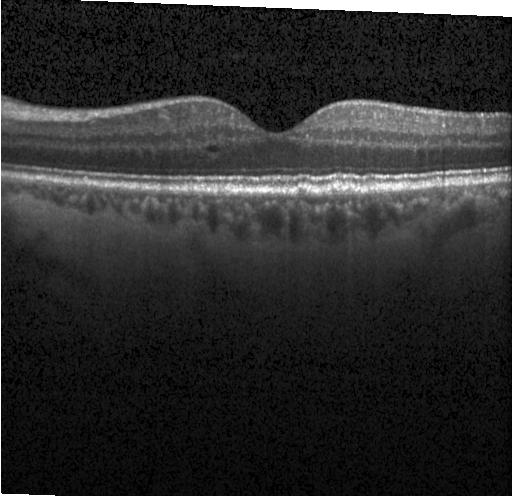

OCT finding: multiple drusen.